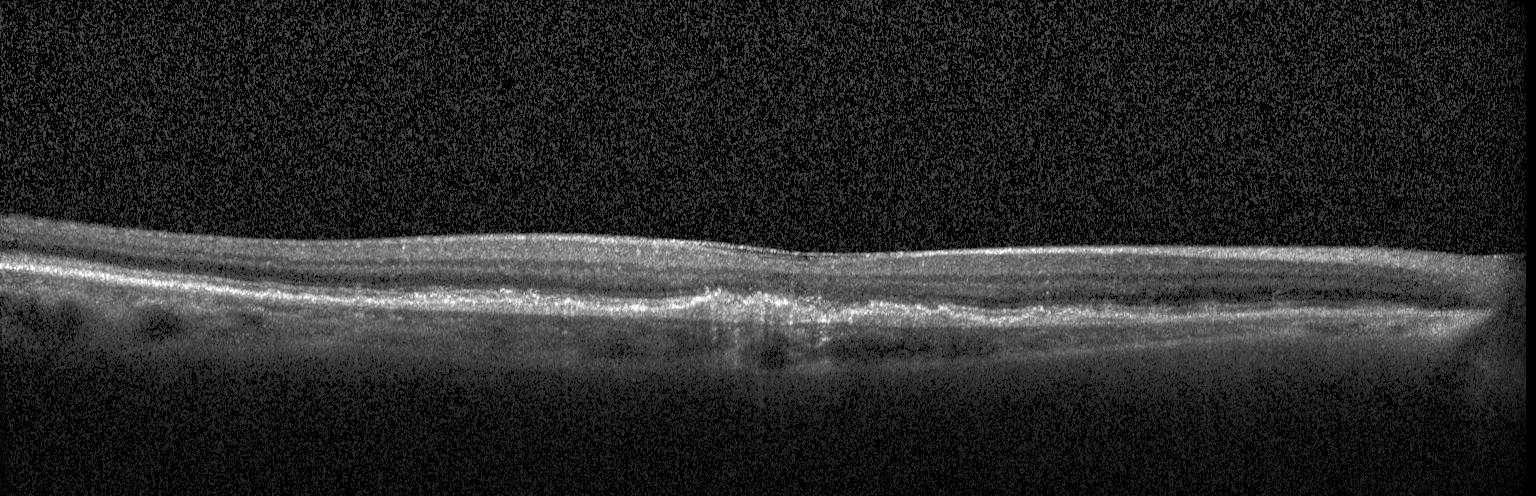
Fovea-centered; Heidelberg Spectralis OCT system; optical coherence tomography B-scan; SD-OCT
Finding: a choroidal neovascular membrane.